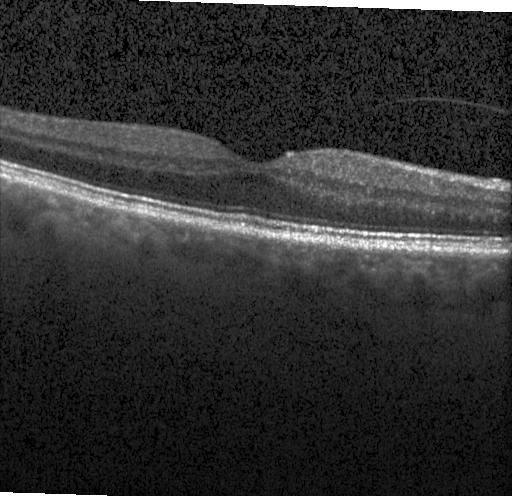 Impression: no choroidal neovascularization, diabetic macular edema, or drusen.